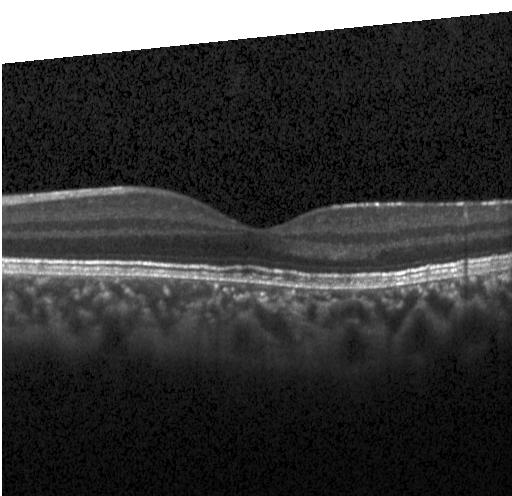

Impression: no CNV, DME, or drusen.